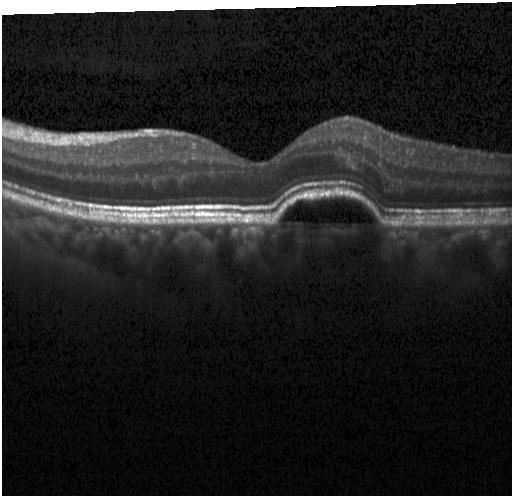

Spectral-domain optical coherence tomography; retinal OCT cross-section. Impression: a choroidal neovascular membrane.